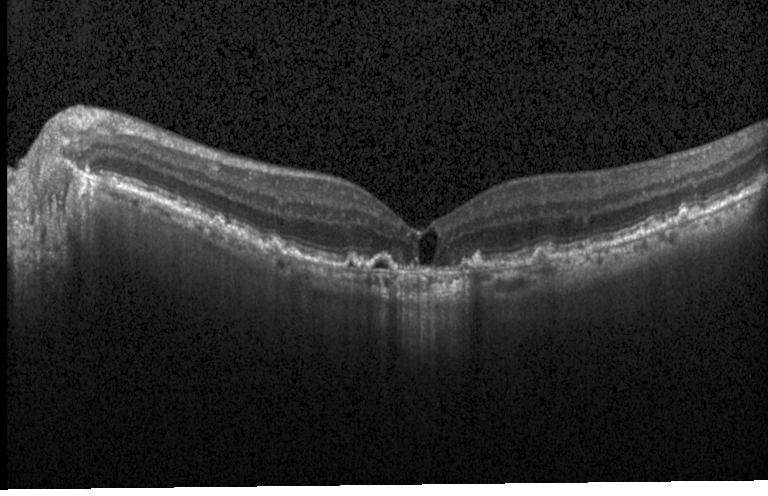
Diagnosis: a choroidal neovascular membrane.